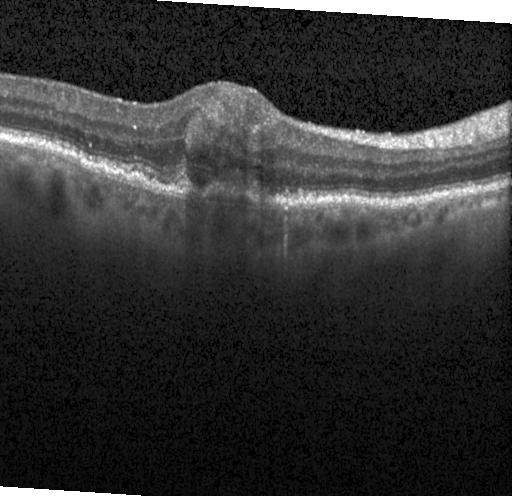

Spectral-domain OCT, optical coherence tomography B-scan, through the macula, Heidelberg Spectralis OCT system. Finding: a choroidal neovascular membrane.